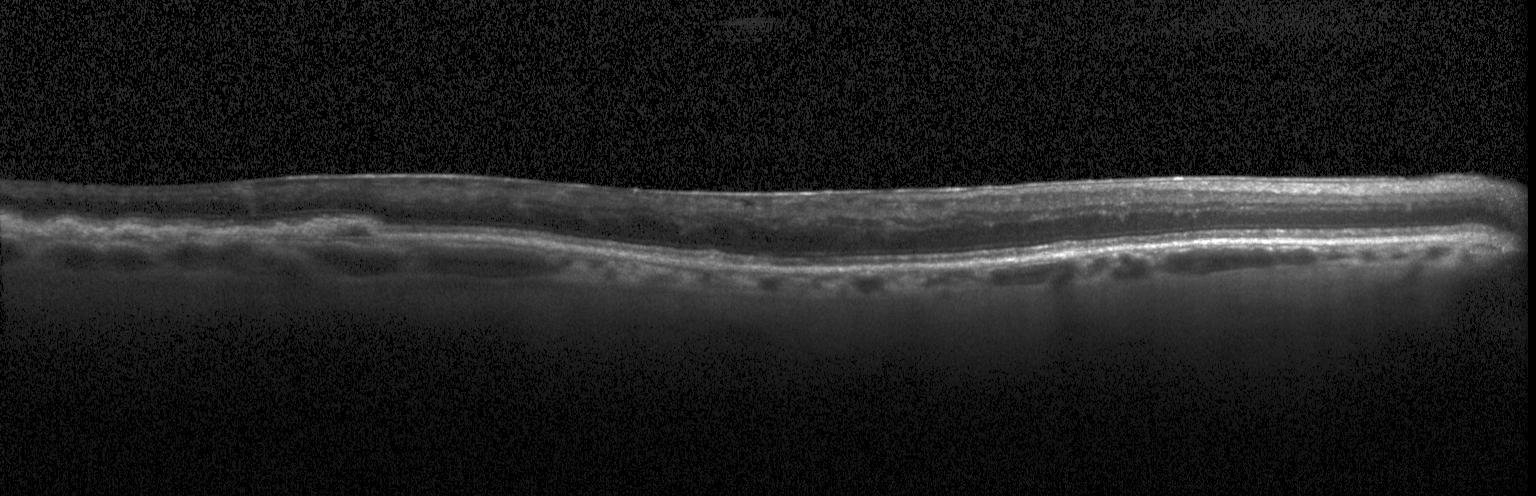

Instrument: Heidelberg Spectralis; optical coherence tomography B-scan — Finding: CNV.